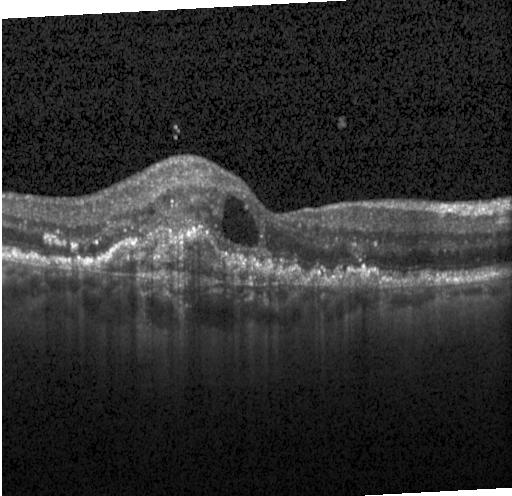
Optical coherence tomography scan. This B-scan demonstrates choroidal neovascularization.